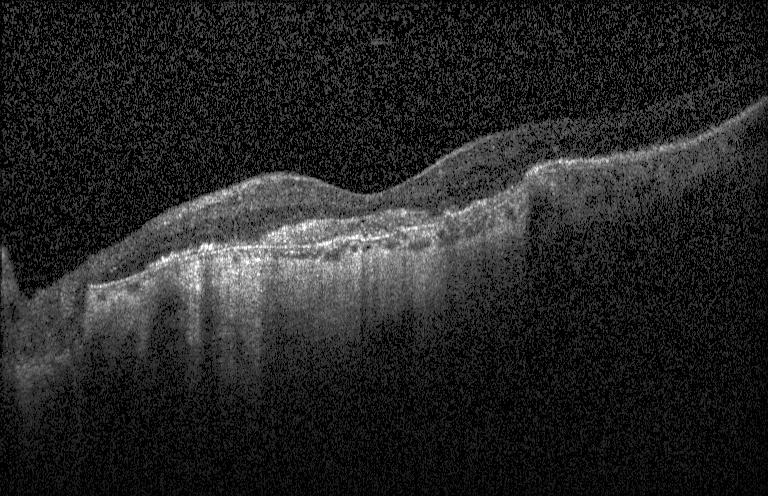 OCT scan showing choroidal neovascularization (CNV).